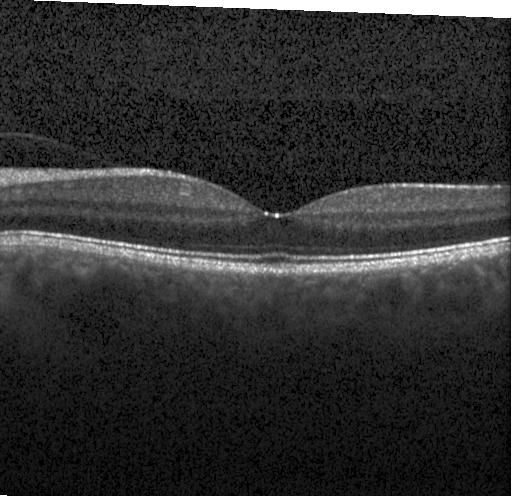

Impression: neither CNV, DME, nor drusen.